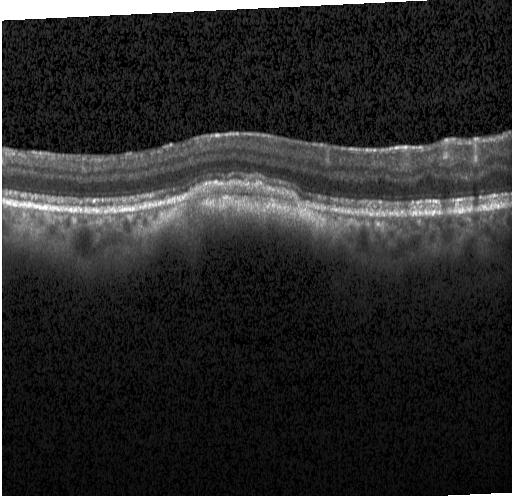 Finding: CNV.